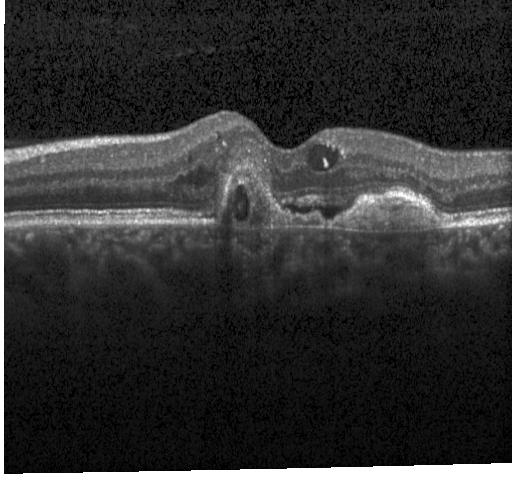 Retinal OCT cross-section showing choroidal neovascularization (CNV).